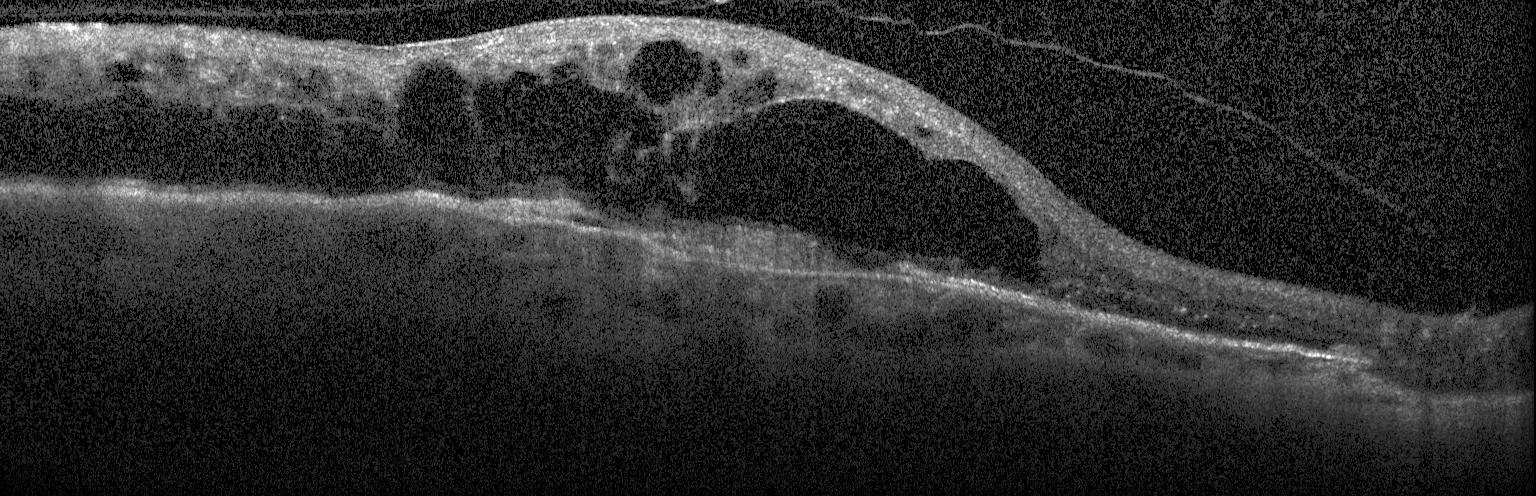
Through the macula · spectral-domain optical coherence tomography · Heidelberg Spectralis · optical coherence tomography B-scan
The scan shows choroidal neovascularization (CNV).